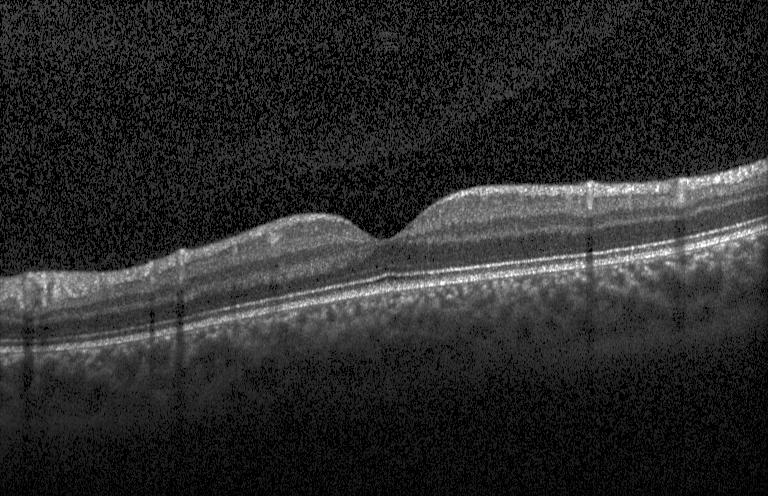

Heidelberg Spectralis OCT system, OCT B-scan, through the macula. Macular OCT: no choroidal neovascularization, no diabetic macular edema, and no drusen.